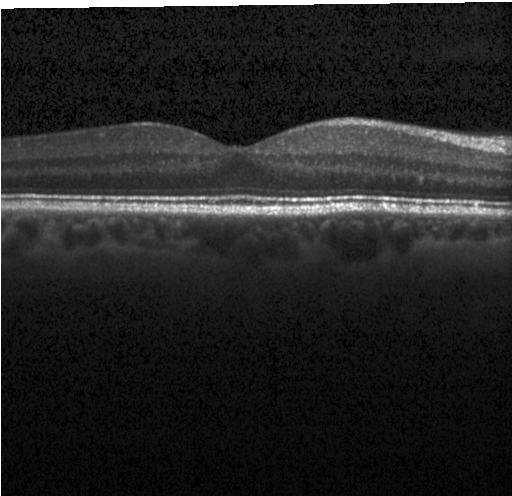

Retinal OCT cross-section showing no evidence of choroidal neovascularization, diabetic macular edema, or drusen.